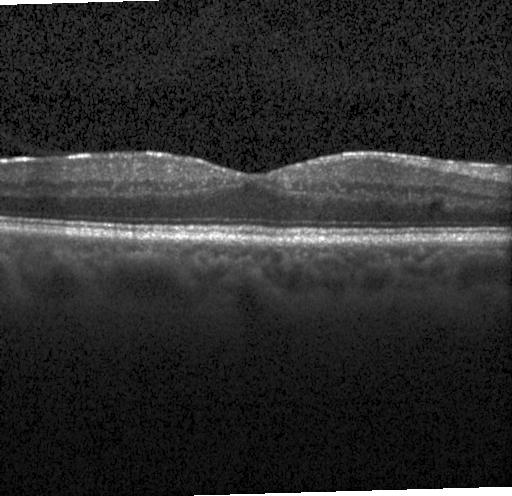
This B-scan demonstrates no choroidal neovascularization, diabetic macular edema, or drusen.